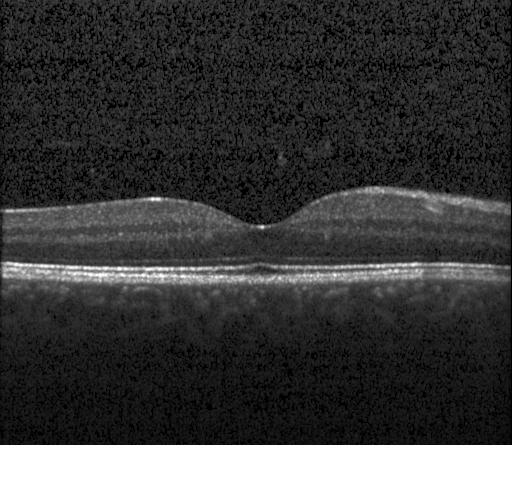 SD-OCT; Heidelberg Spectralis OCT system; optical coherence tomography B-scan — Finding: no evidence of choroidal neovascularization, diabetic macular edema, or drusen.